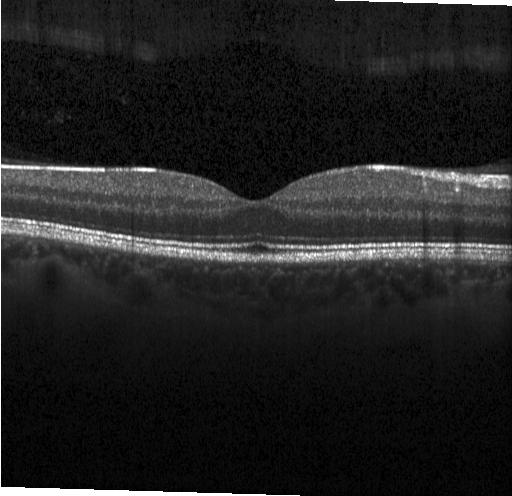
Spectral-domain optical coherence tomography · optical coherence tomography B-scan · instrument: Heidelberg Spectralis.
Diagnosis: no choroidal neovascularization, no diabetic macular edema, and no drusen.